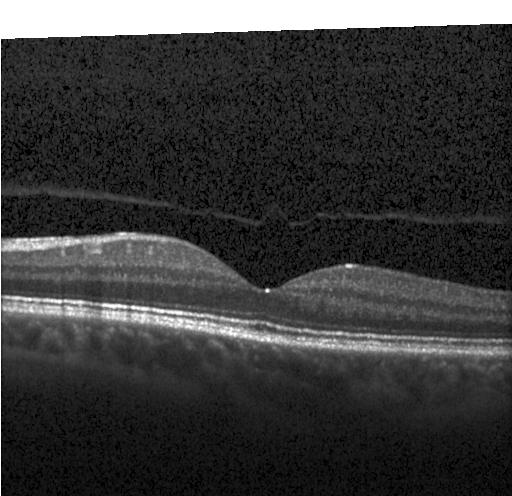
Horizontal scan through the fovea. SD-OCT. Optical coherence tomography B-scan.
OCT finding: no evidence of choroidal neovascularization, diabetic macular edema, or drusen.